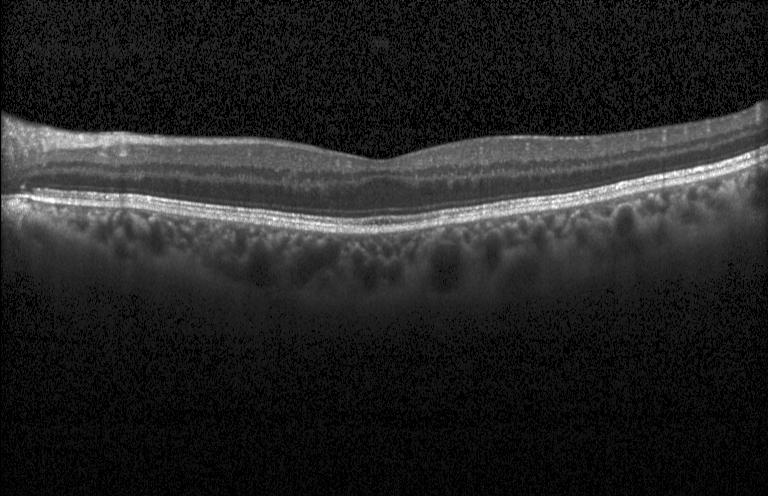 Finding: no choroidal neovascularization, diabetic macular edema, or drusen.